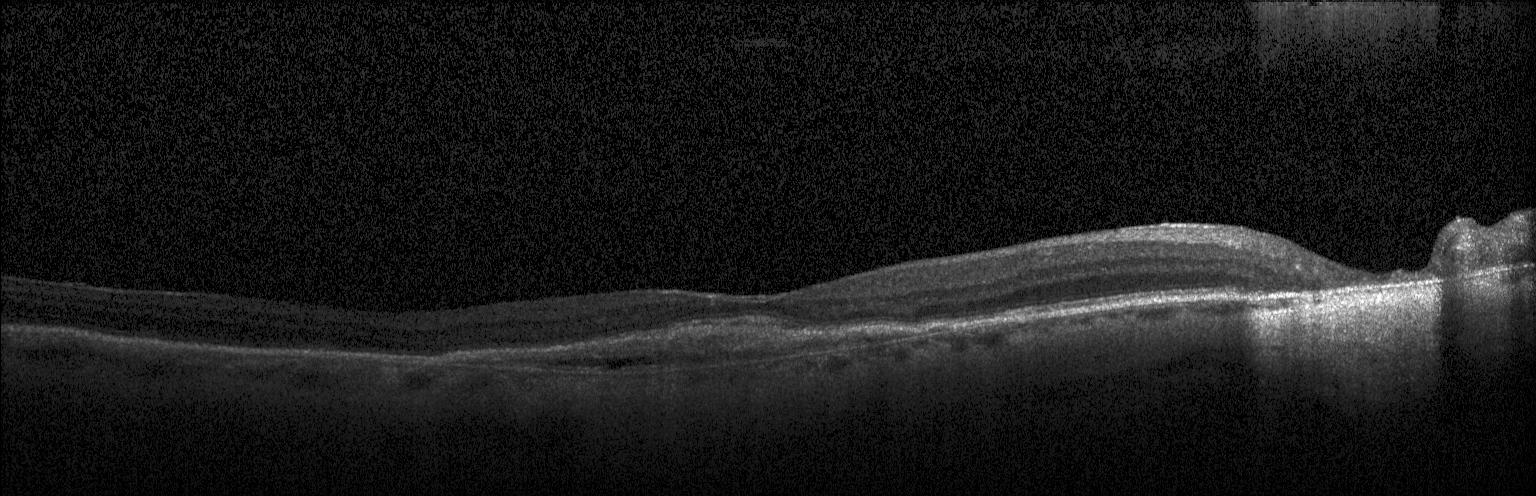

Retinal OCT B-scan — Finding: choroidal neovascularization.